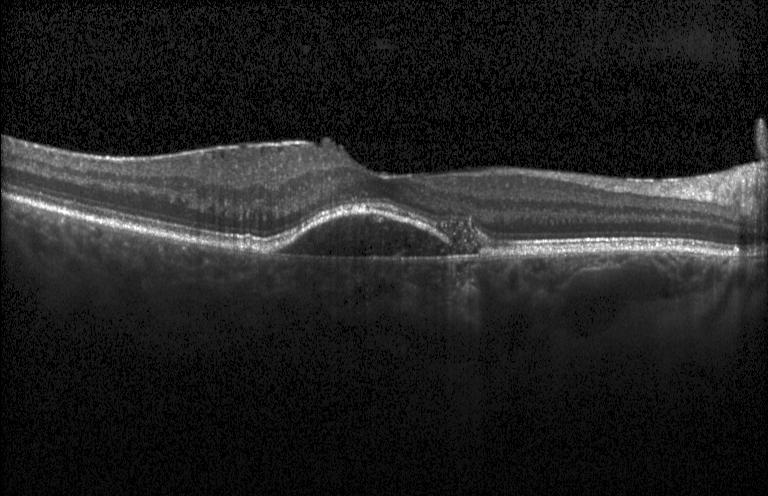

Macular scan; optical coherence tomography scan.
This B-scan demonstrates a choroidal neovascular membrane.